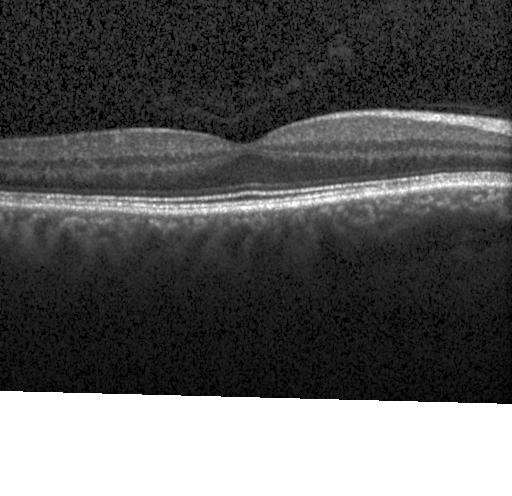

Retinal OCT B-scan; spectral-domain OCT
Finding: no CNV, DME, or drusen.